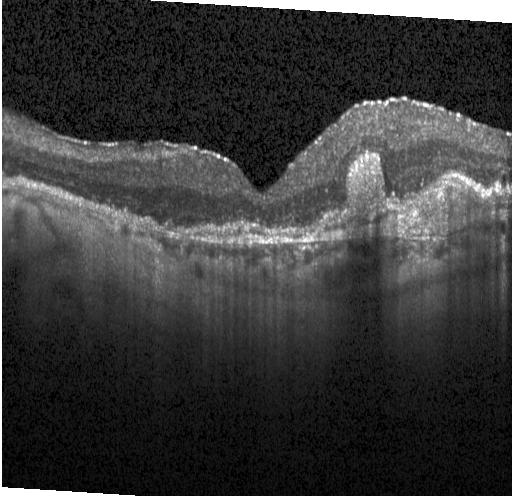
SD-OCT, optical coherence tomography scan, horizontal scan through the fovea, Heidelberg Spectralis OCT system.
Diagnosis: choroidal neovascularization.